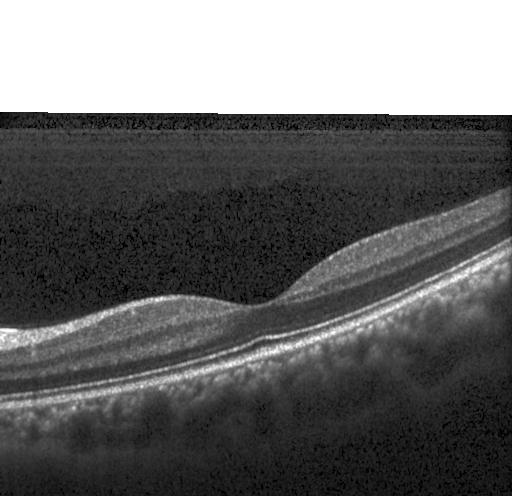 OCT B-scan. Macular scan. Heidelberg Spectralis.
Finding: no CNV, DME, or drusen.